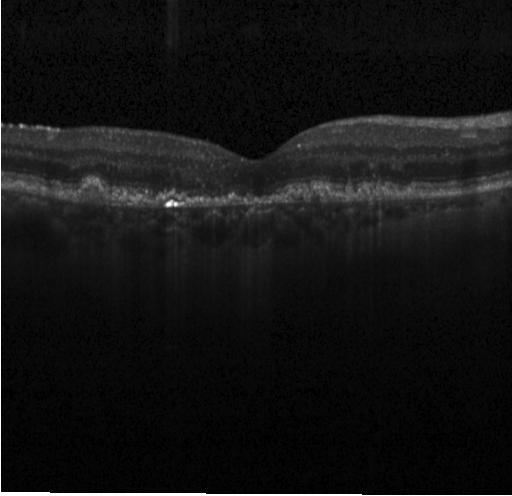
Optical coherence tomography B-scan · acquired on a Heidelberg Spectralis. A choroidal neovascular membrane.